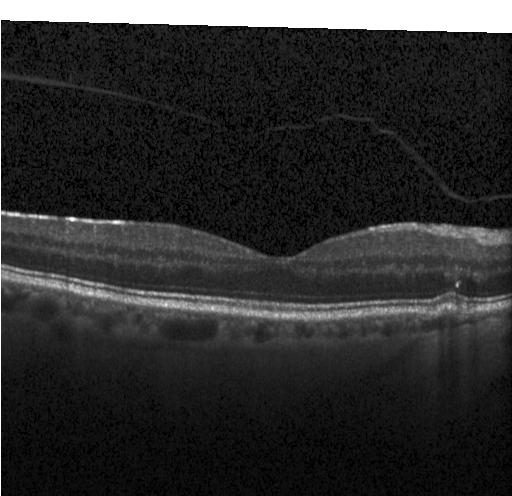

OCT B-scan. Spectral-domain OCT. Impression: drusen.